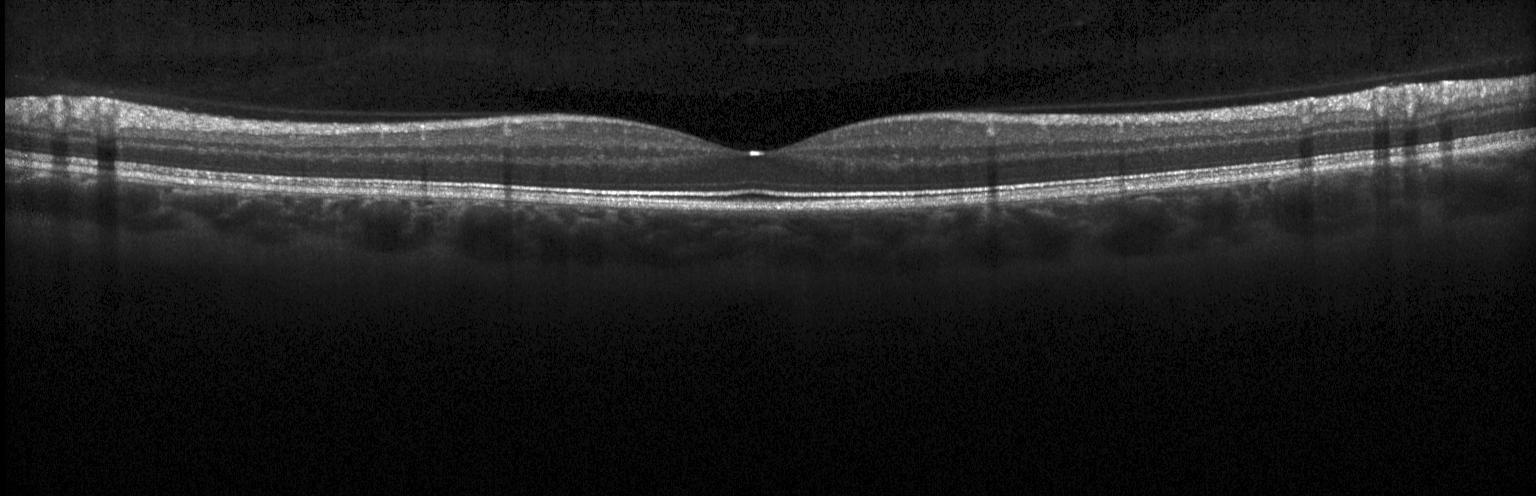 SD-OCT · fovea-centered · acquired on a Heidelberg Spectralis · retinal OCT cross-section
Dx: neither choroidal neovascularization, diabetic macular edema, nor drusen.